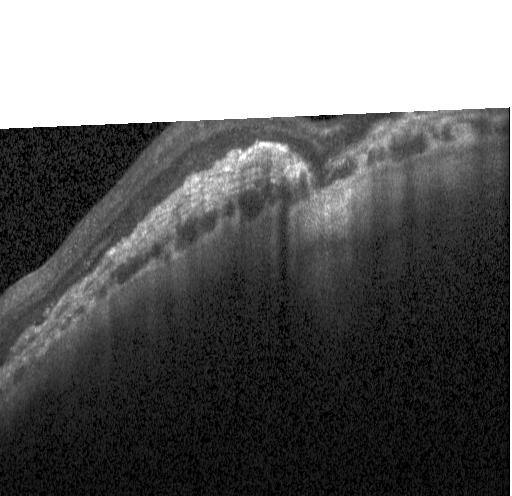 Diagnosis: CNV.